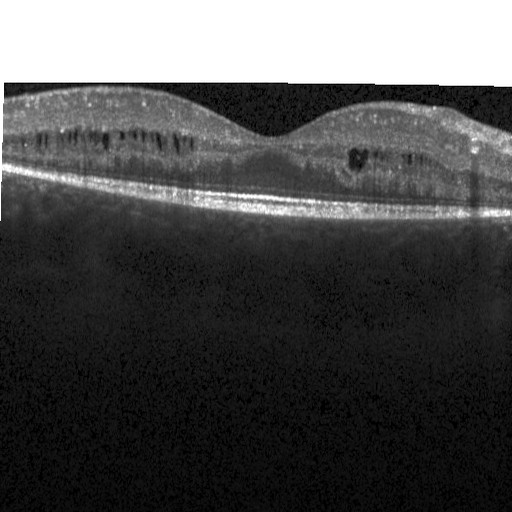
Acquired on a Heidelberg Spectralis; SD-OCT; OCT B-scan; fovea-centered
The scan shows diabetic macular edema.